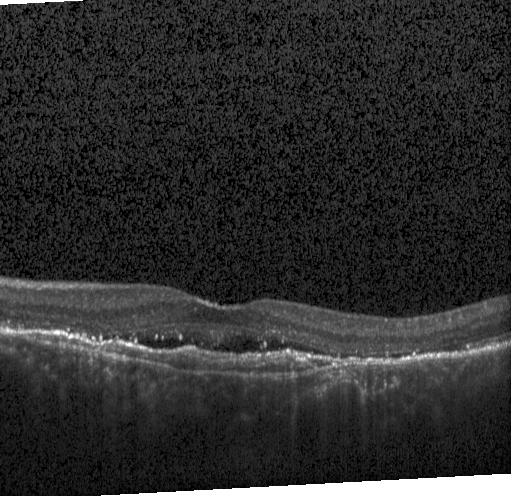

Impression: choroidal neovascularization.